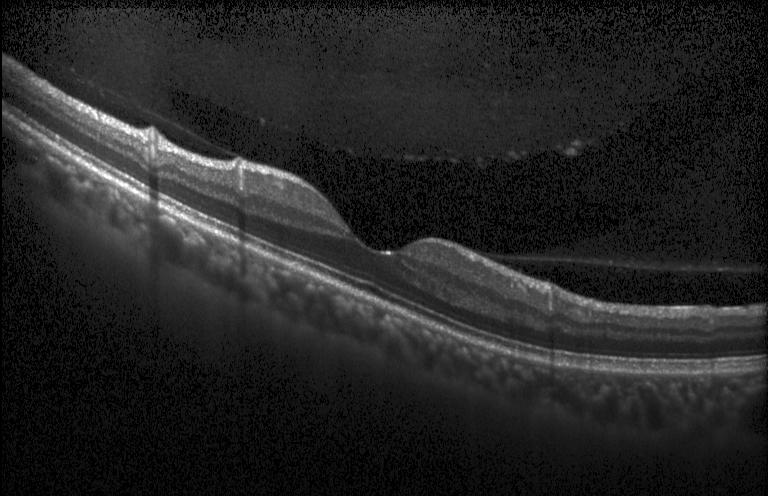
Neither choroidal neovascularization, diabetic macular edema, nor drusen.